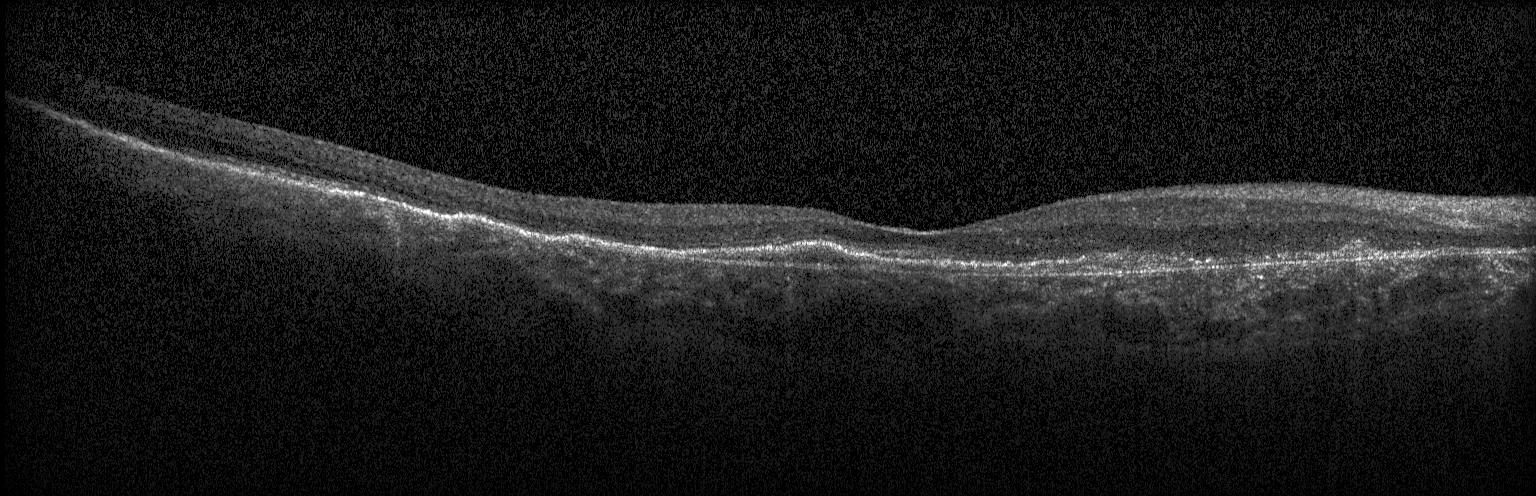
Finding: choroidal neovascularization.